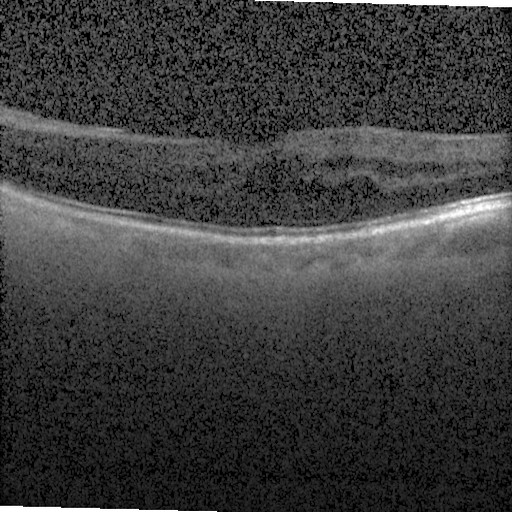

Finding: diabetic macular edema (DME).